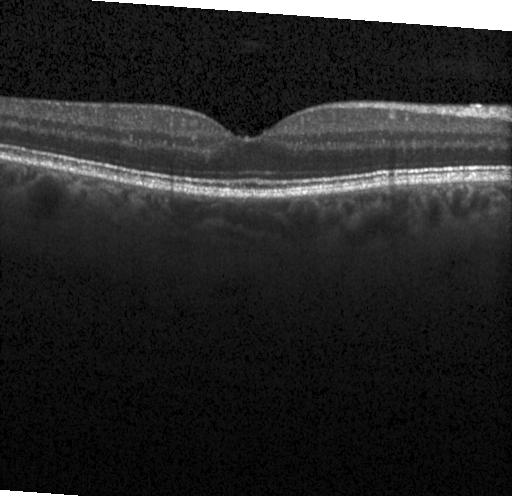 SD-OCT. Centered on the fovea. Optical coherence tomography B-scan.
Impression: no CNV, DME, or drusen.